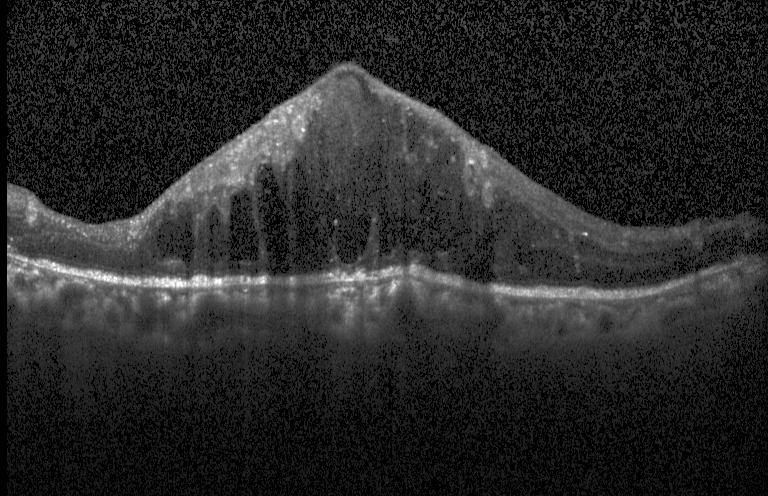 Heidelberg Spectralis OCT system. SD-OCT. Centered on the fovea. Retinal OCT cross-section — Finding: diabetic macular edema (DME).